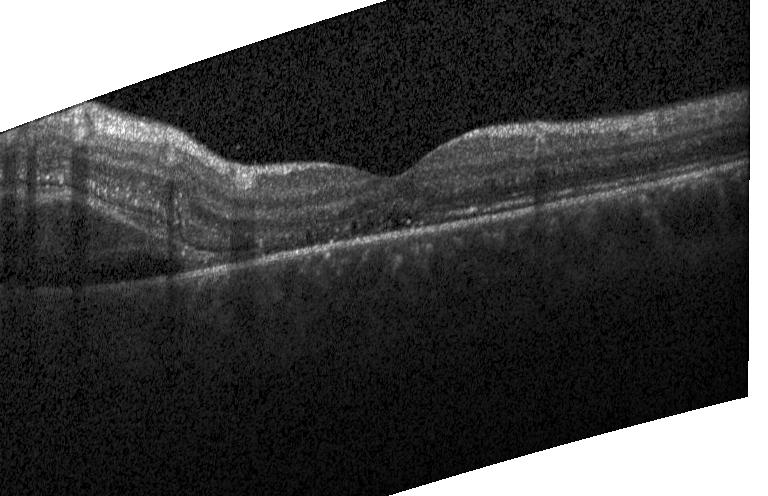

SD-OCT, Heidelberg Spectralis OCT system, optical coherence tomography scan, fovea-centered
Finding: a choroidal neovascular membrane.